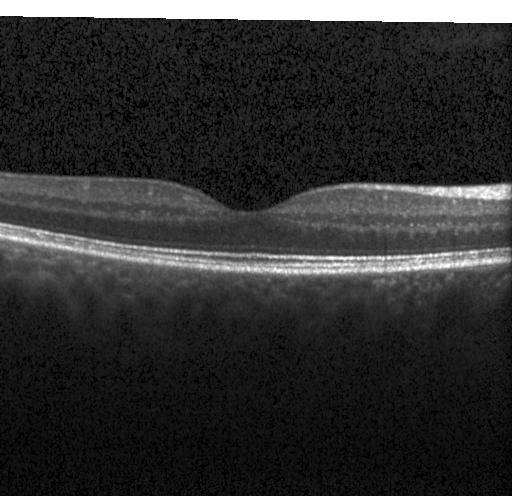

Finding: neither choroidal neovascularization, diabetic macular edema, nor drusen.